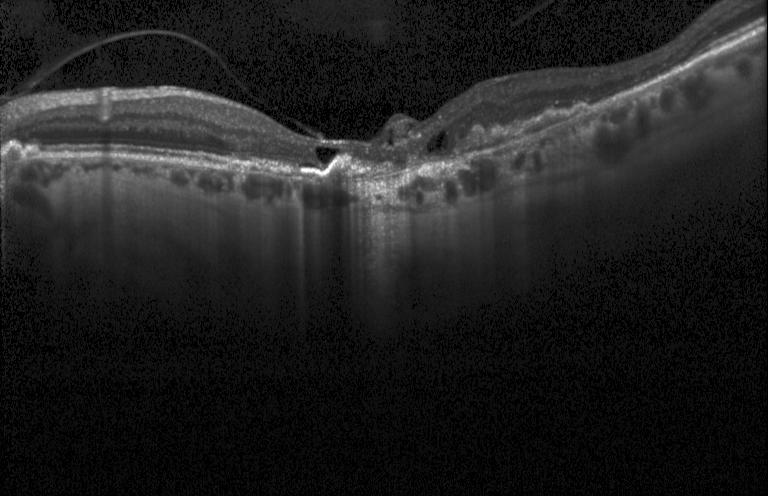
Impression: choroidal neovascularization (CNV).